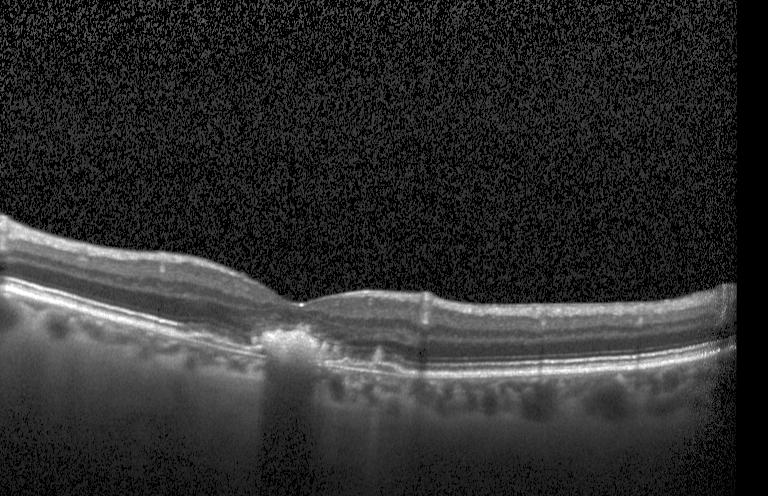 Optical coherence tomography scan · SD-OCT · fovea-centered · Heidelberg Spectralis OCT system
Diagnosis: choroidal neovascularization.